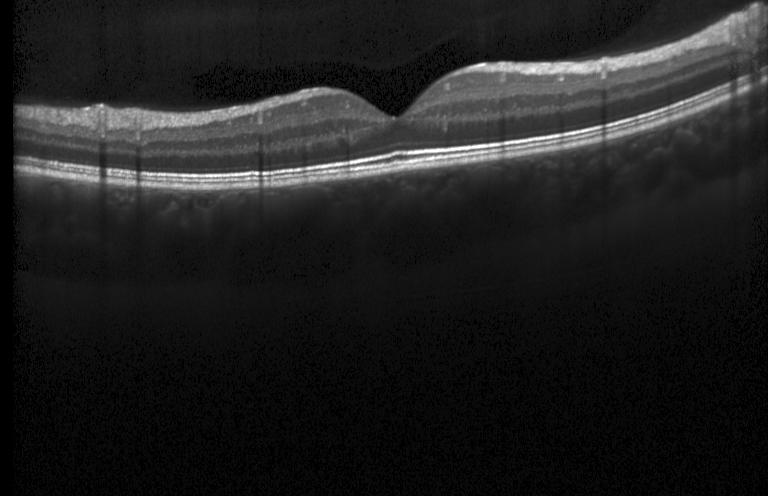 SD-OCT; optical coherence tomography B-scan; Heidelberg Spectralis OCT system; centered on the fovea — Dx: neither CNV, DME, nor drusen.